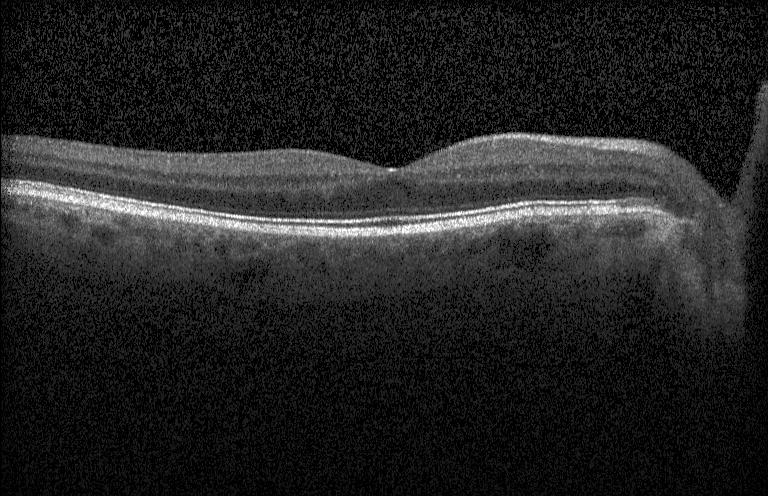

OCT B-scan showing no choroidal neovascularization, diabetic macular edema, or drusen.